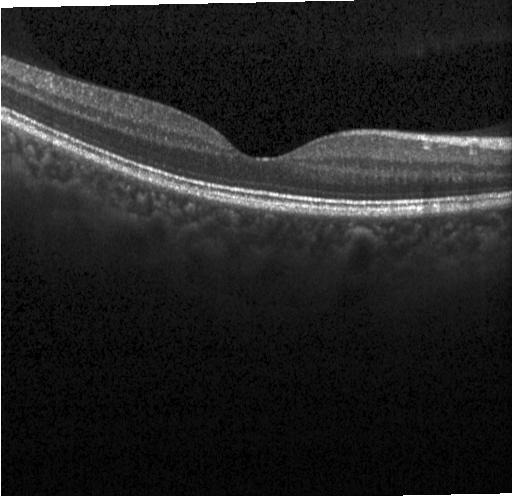

OCT B-scan showing no CNV, DME, or drusen.